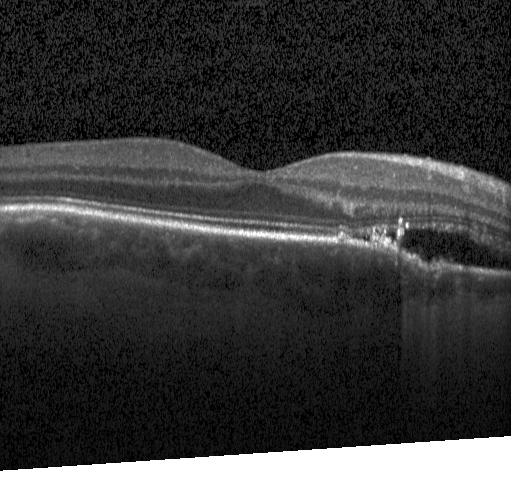
Horizontal scan through the fovea, optical coherence tomography scan, spectral-domain optical coherence tomography — Dx: a choroidal neovascular membrane.